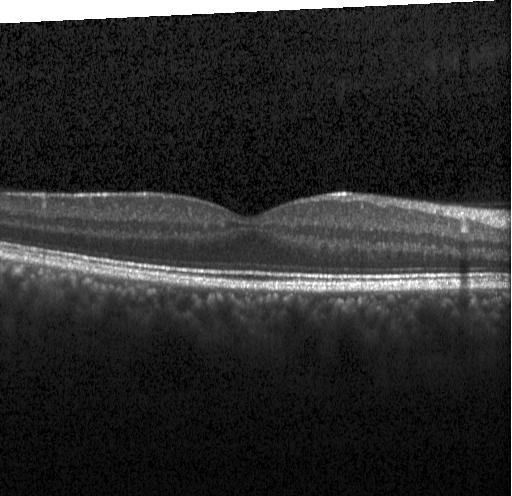
Dx: neither CNV, DME, nor drusen.